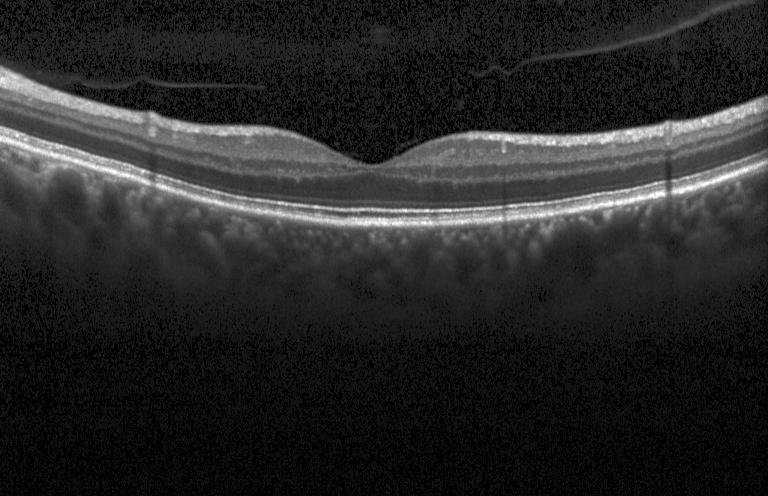 No CNV, DME, or drusen.